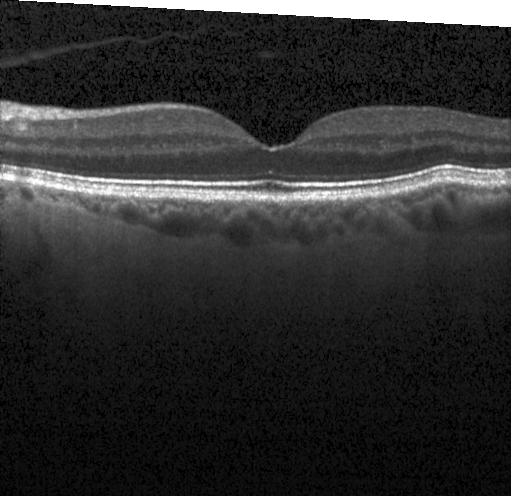
OCT line scan · Heidelberg Spectralis OCT system · horizontal scan through the fovea · spectral-domain OCT
Impression: no CNV, no DME, and no drusen.